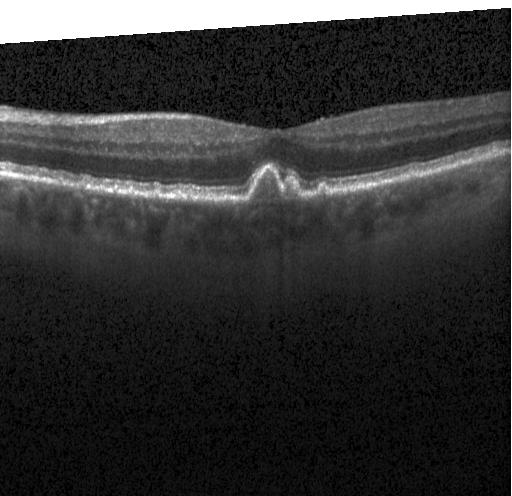
OCT B-scan, horizontal scan through the fovea — Assessment: multiple drusen.